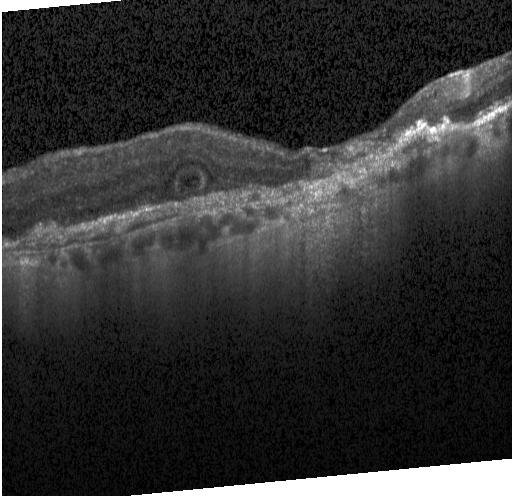
Through the macula, Heidelberg Spectralis, spectral-domain OCT, optical coherence tomography scan — This B-scan demonstrates a choroidal neovascular membrane.